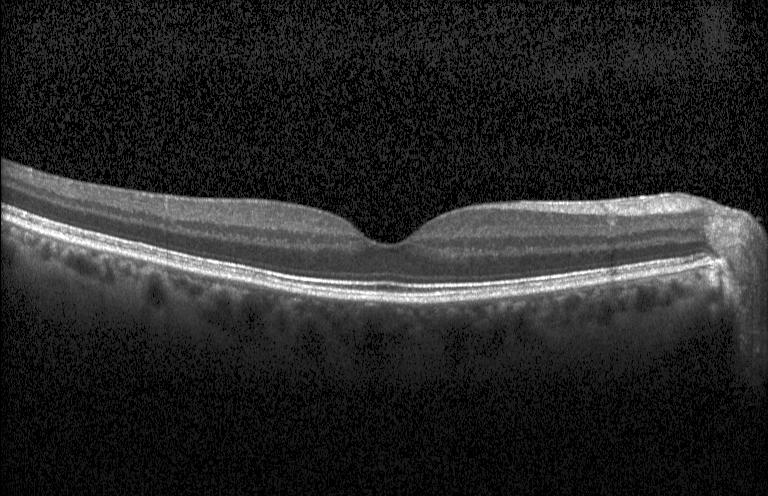 Through the macula, spectral-domain optical coherence tomography, OCT line scan
Impression: no evidence of choroidal neovascularization, diabetic macular edema, or drusen.